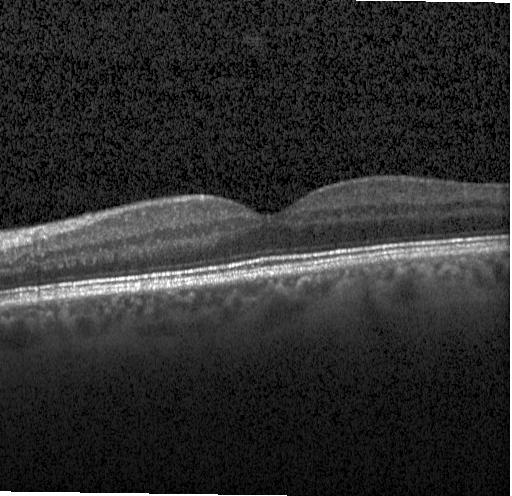
Optical coherence tomography B-scan; fovea-centered; Heidelberg Spectralis
This B-scan demonstrates no choroidal neovascularization, diabetic macular edema, or drusen.